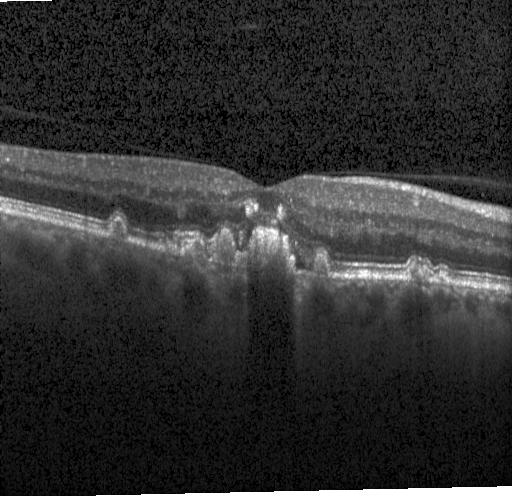
Diagnosis: a choroidal neovascular membrane.